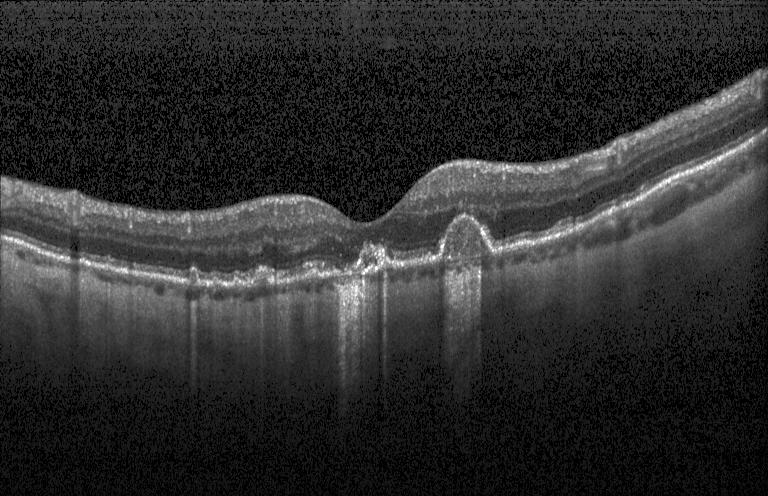
Spectral-domain optical coherence tomography; optical coherence tomography scan.
Finding: choroidal neovascularization (CNV).